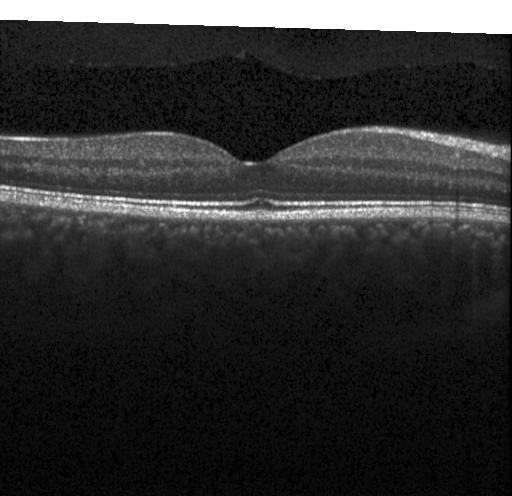
OCT B-scan.
Impression: no CNV, no DME, and no drusen.